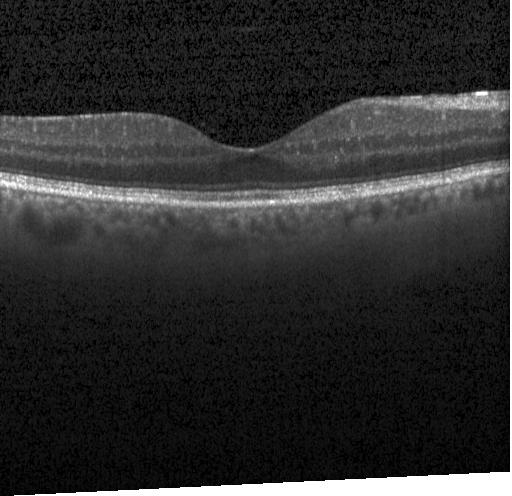 Macular OCT demonstrating no evidence of choroidal neovascularization, diabetic macular edema, or drusen.